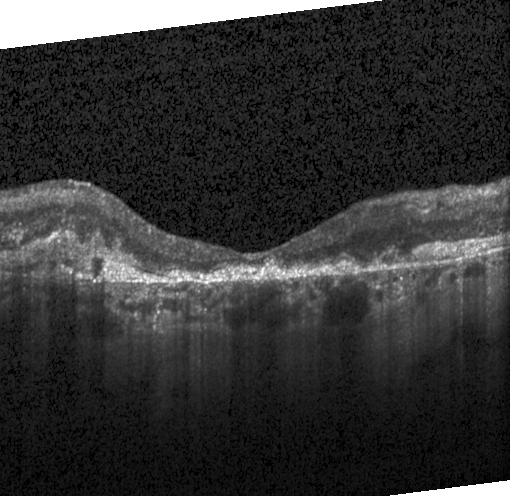

Retinal OCT B-scan. Centered on the fovea — Dx: a choroidal neovascular membrane.